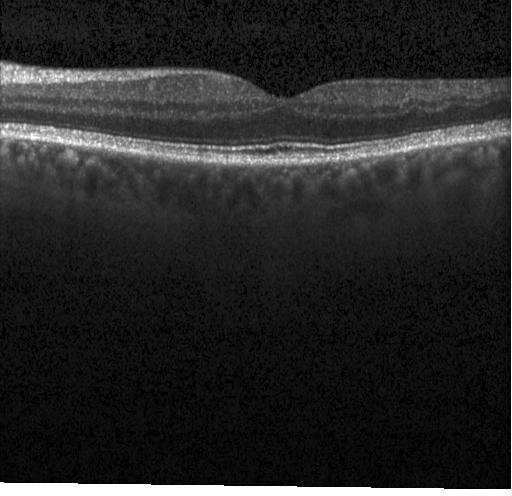

Instrument: Heidelberg Spectralis; horizontal scan through the fovea; spectral-domain OCT; retinal OCT cross-section.
Diagnosis: neither choroidal neovascularization, diabetic macular edema, nor drusen.